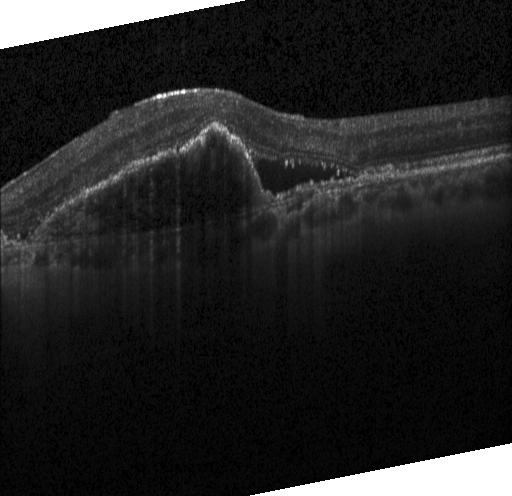 Horizontal scan through the fovea. Heidelberg Spectralis OCT system. Retinal OCT B-scan
Diagnosis: a choroidal neovascular membrane.